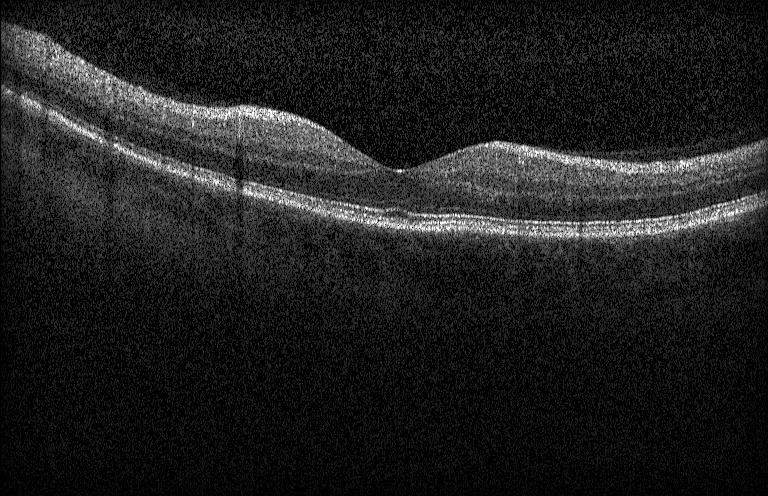
OCT B-scan — Finding: no evidence of CNV, DME, or drusen.